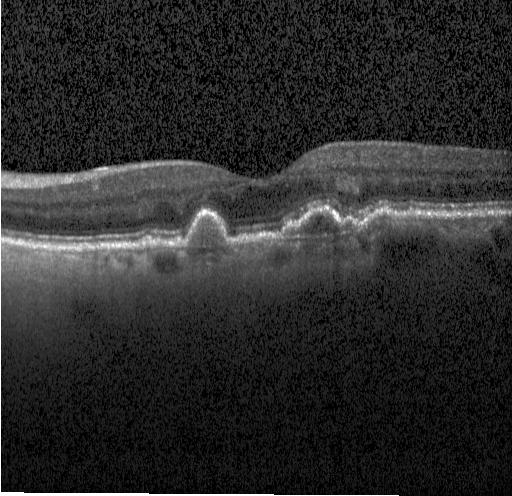

The scan shows choroidal neovascularization (CNV).